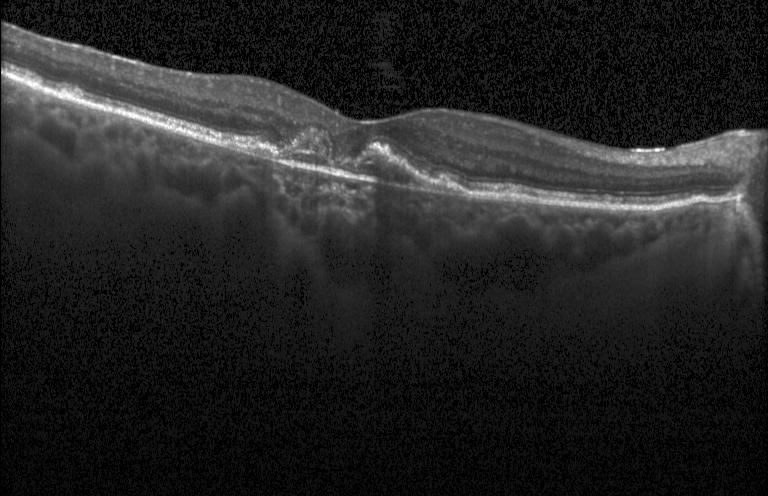 The scan shows a choroidal neovascular membrane.